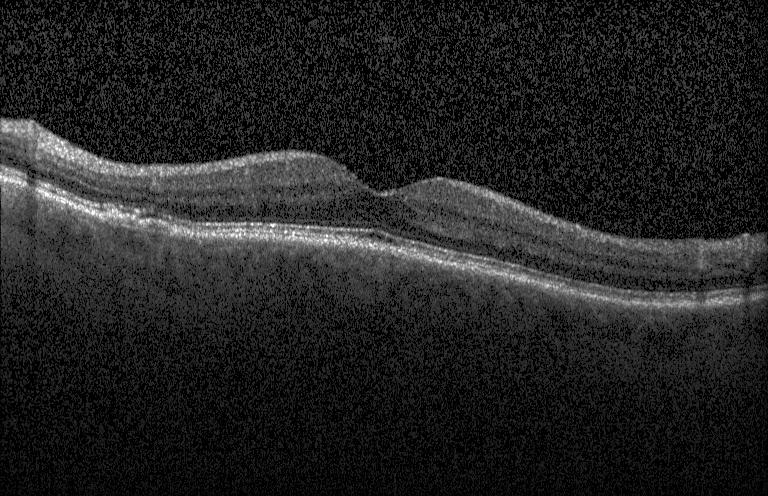
Finding: choroidal neovascularization.